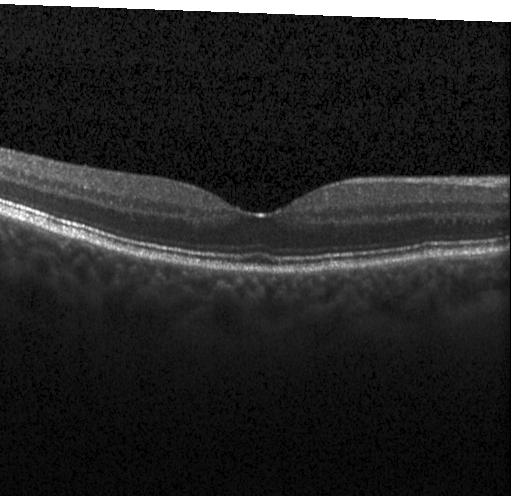
Retinal OCT B-scan.
Assessment: no choroidal neovascularization, no diabetic macular edema, and no drusen.